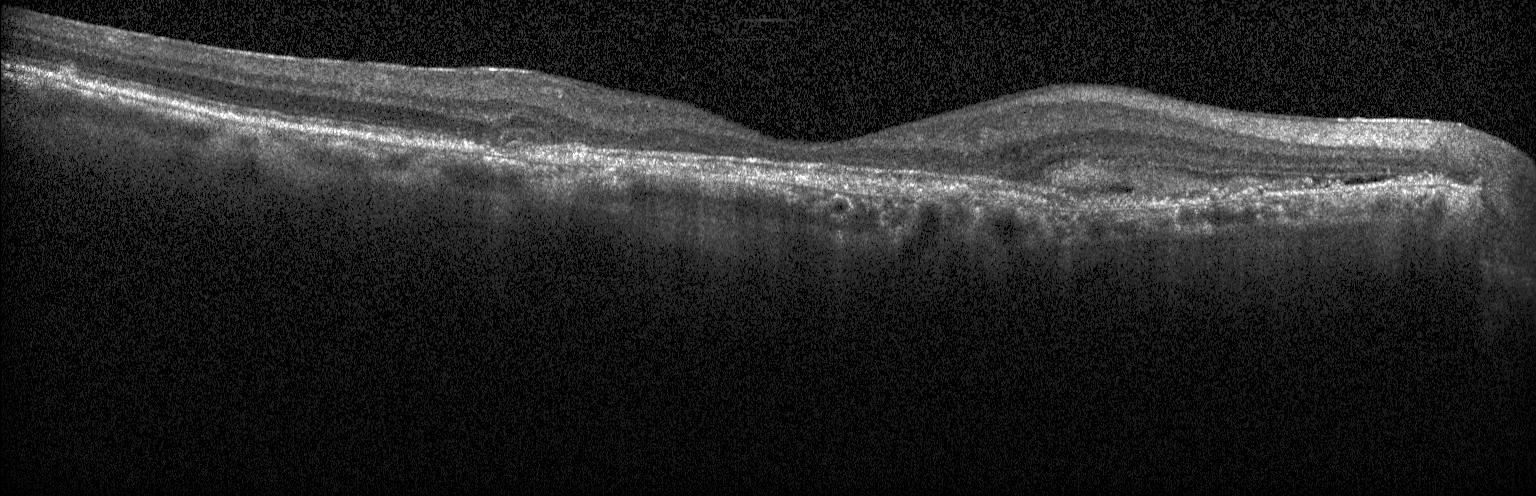
SD-OCT, retinal OCT cross-section — Choroidal neovascularization (CNV).